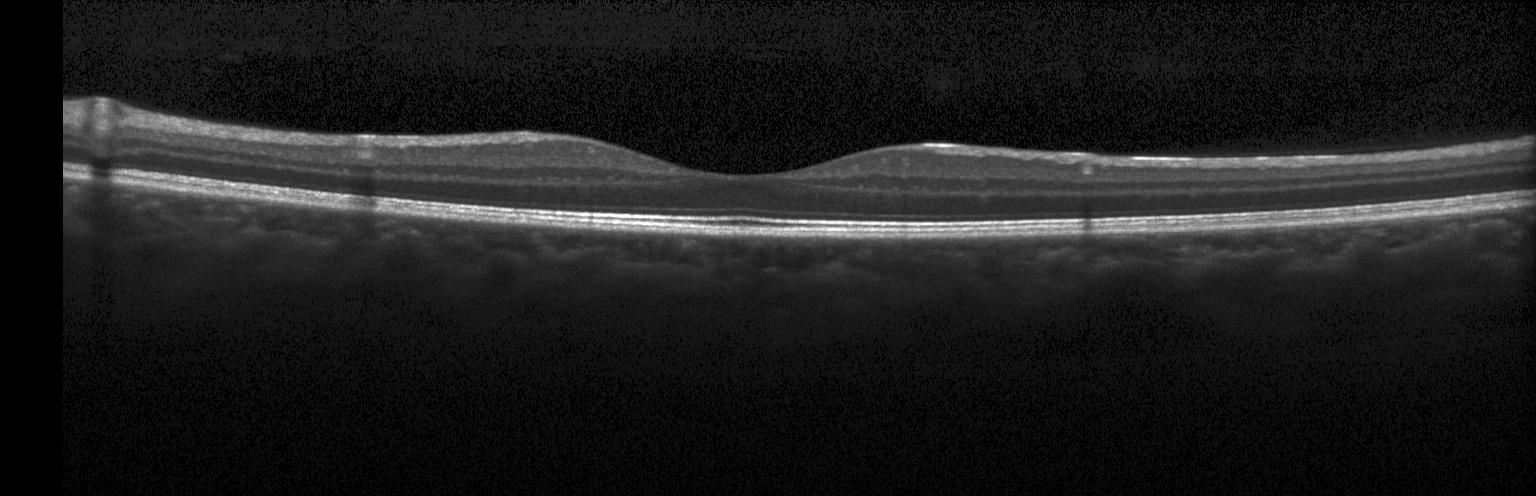

OCT line scan, macular scan, Heidelberg Spectralis OCT system, SD-OCT — The scan shows neither choroidal neovascularization, diabetic macular edema, nor drusen.